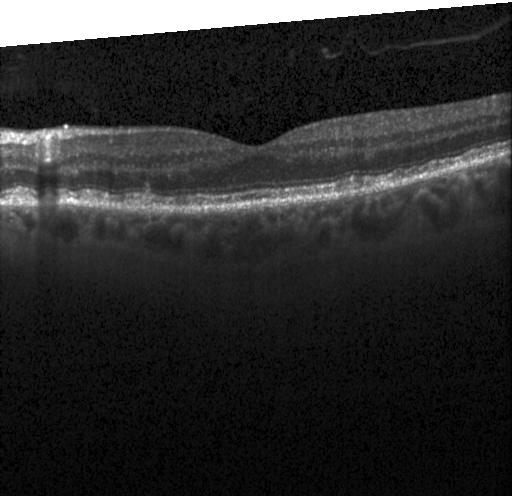
OCT line scan.
Finding: drusen.